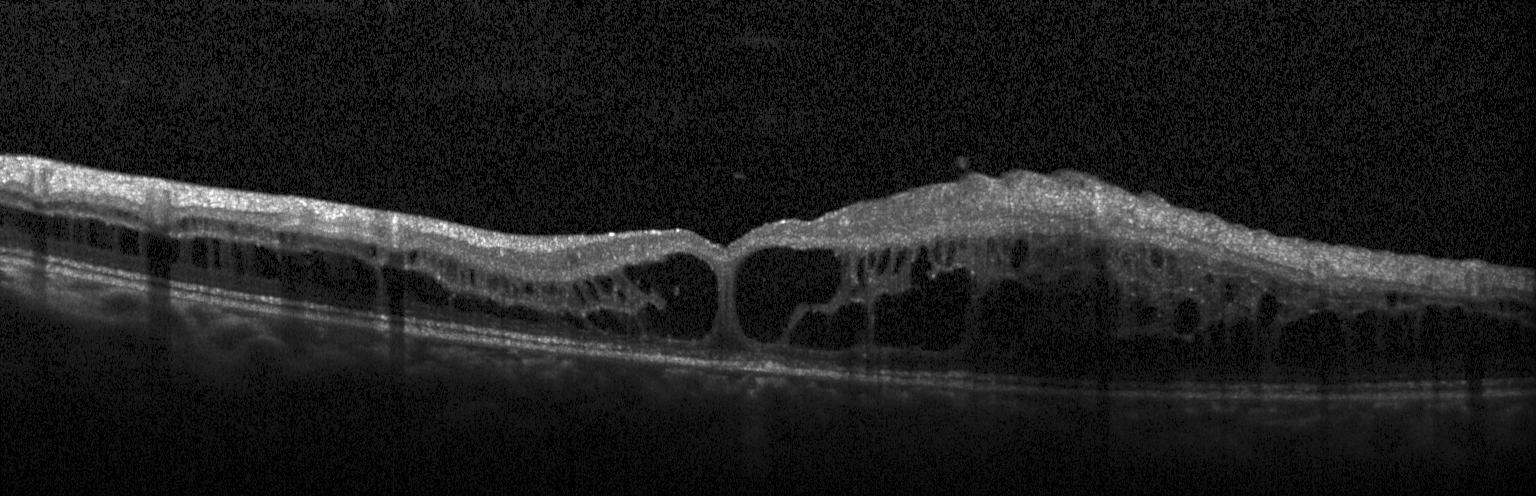
OCT line scan — This B-scan demonstrates DME.